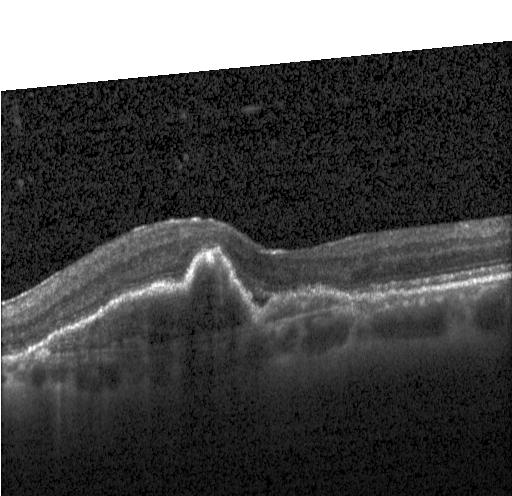 OCT B-scan, Heidelberg Spectralis.
Finding: a choroidal neovascular membrane.